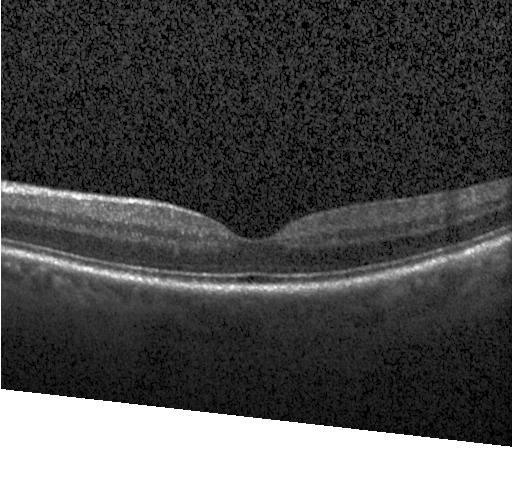 Spectral-domain OCT · retinal OCT B-scan · macular scan · acquired on a Heidelberg Spectralis. OCT finding: no choroidal neovascularization, no diabetic macular edema, and no drusen.